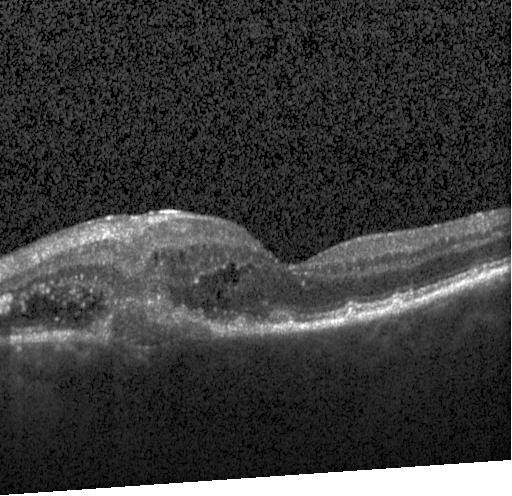
Centered on the fovea; retinal OCT B-scan — Assessment: a choroidal neovascular membrane.